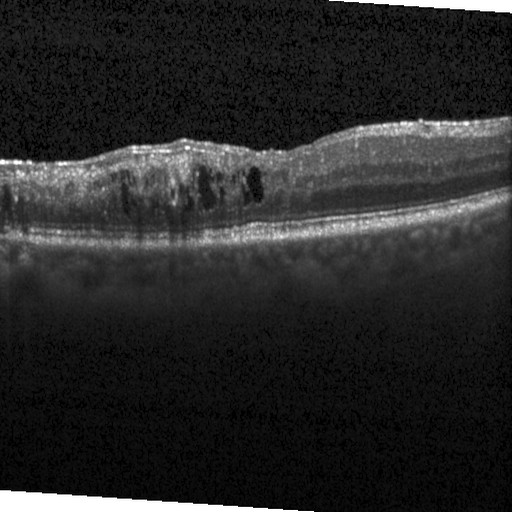 OCT line scan. Fovea-centered. SD-OCT
Diagnosis: diabetic macular edema.